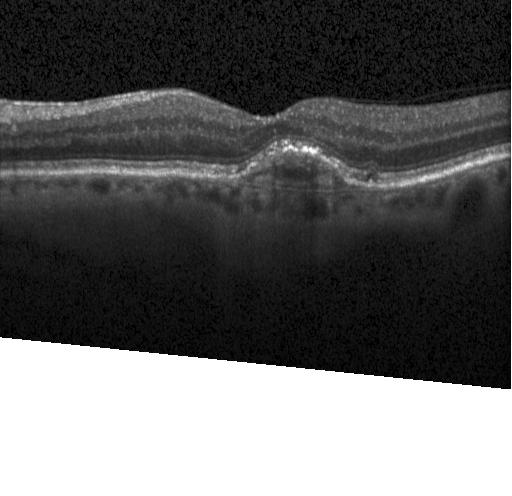 Optical coherence tomography scan. OCT finding: a choroidal neovascular membrane.